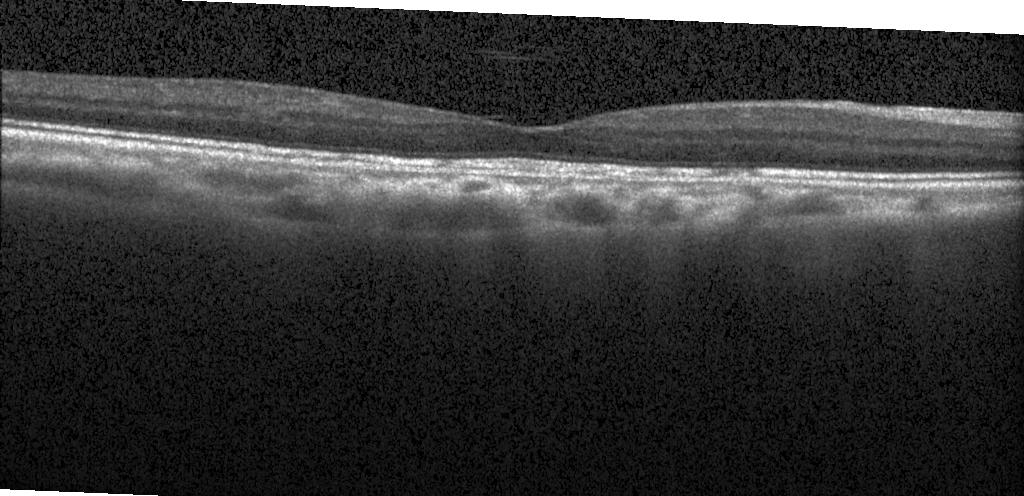 Dx: no evidence of CNV, DME, or drusen.